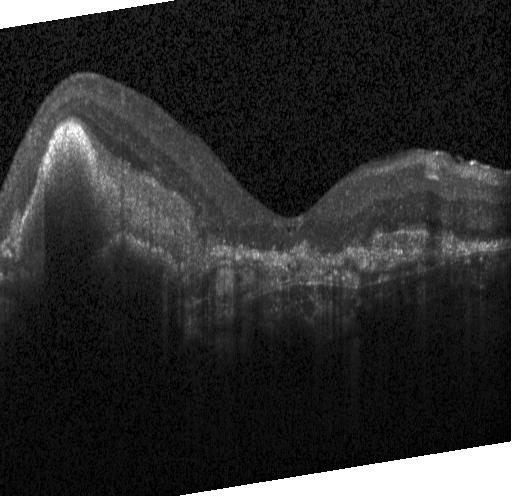
Heidelberg Spectralis OCT system; spectral-domain OCT; centered on the fovea; optical coherence tomography scan — Macular OCT: a choroidal neovascular membrane.